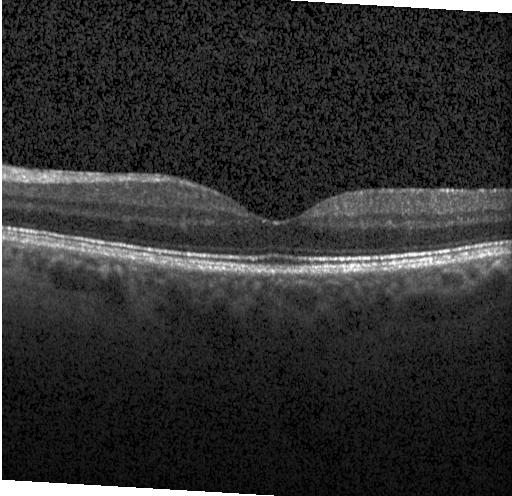 Finding: no choroidal neovascularization, diabetic macular edema, or drusen.